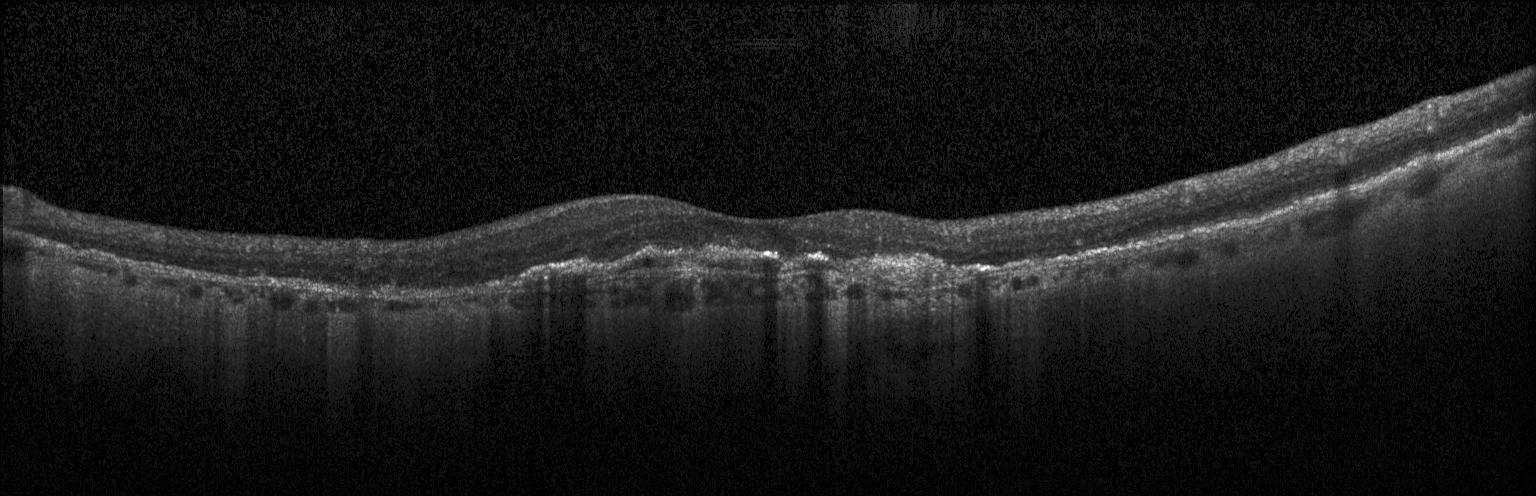
This B-scan demonstrates choroidal neovascularization (CNV).